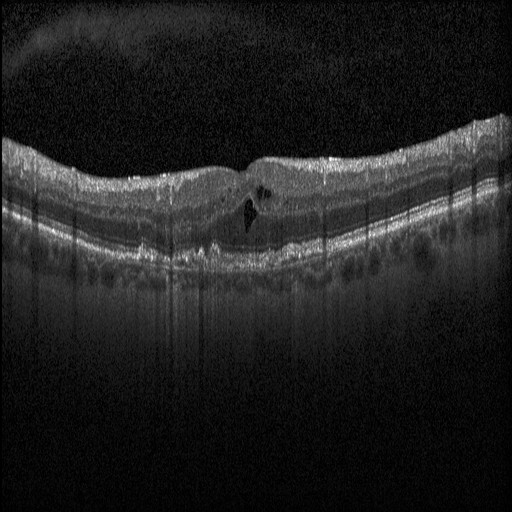
Spectral-domain OCT · through the macula · retinal OCT B-scan — Finding: diabetic macular edema (DME).